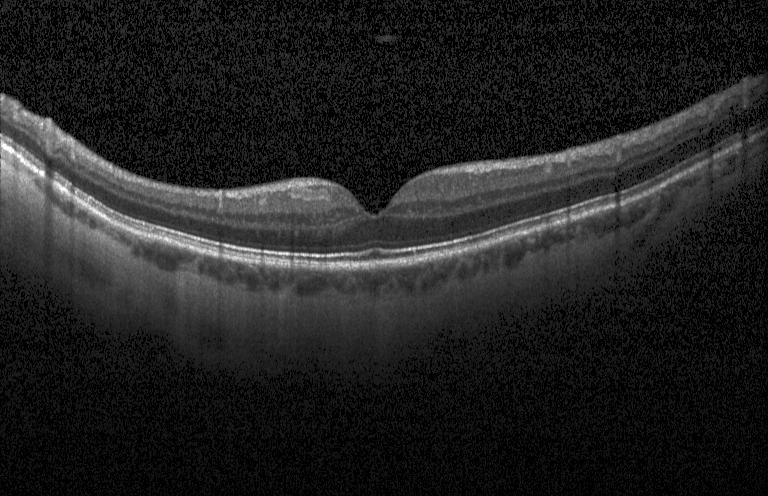 Retinal OCT B-scan · spectral-domain optical coherence tomography · acquired on a Heidelberg Spectralis — Impression: no CNV, no DME, and no drusen.